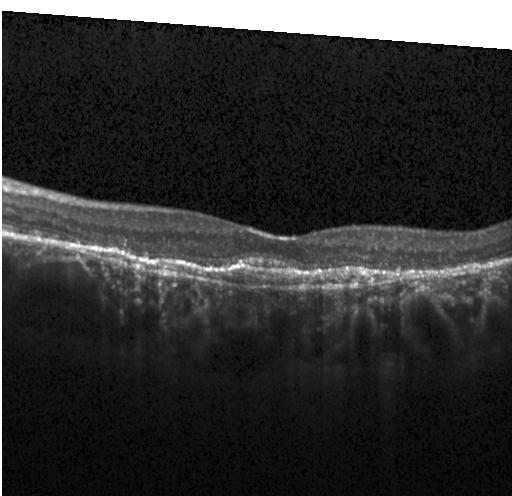
Spectral-domain optical coherence tomography, retinal OCT cross-section. This B-scan demonstrates choroidal neovascularization.